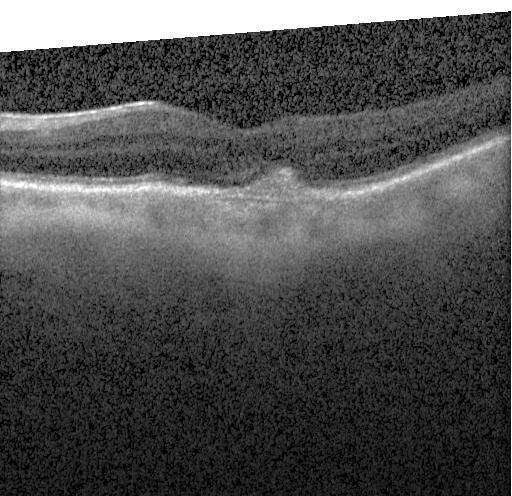 OCT finding: choroidal neovascularization (CNV).